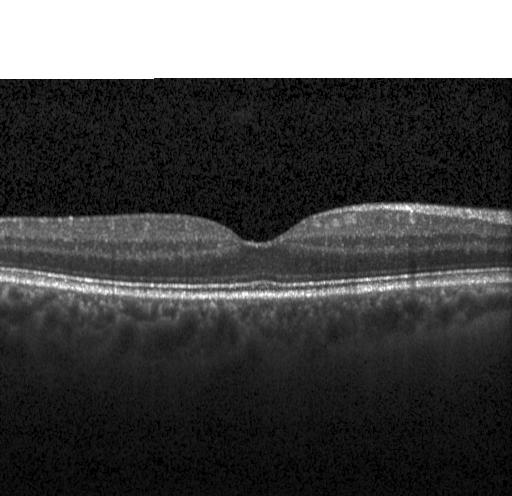

Finding: no evidence of choroidal neovascularization, diabetic macular edema, or drusen.